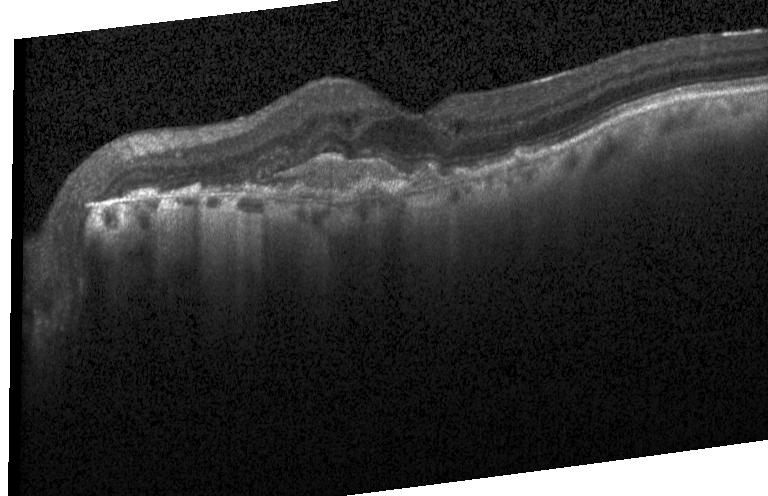 Retinal OCT B-scan. Spectral-domain optical coherence tomography. Instrument: Heidelberg Spectralis. Macular scan.
Dx: CNV.